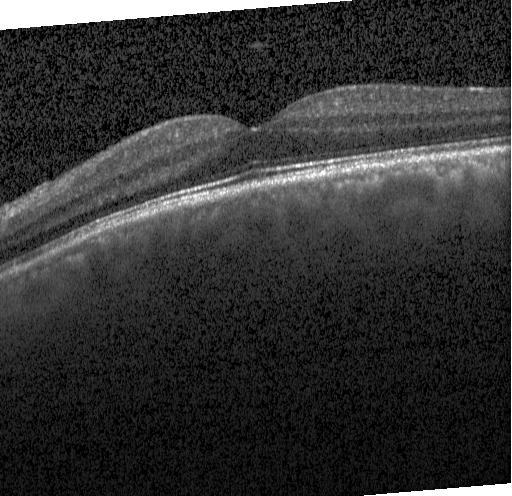

OCT B-scan showing no choroidal neovascularization, diabetic macular edema, or drusen.